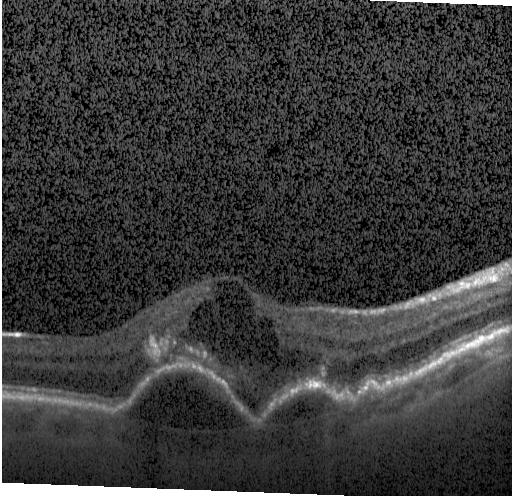 Optical coherence tomography B-scan — Dx: a choroidal neovascular membrane.